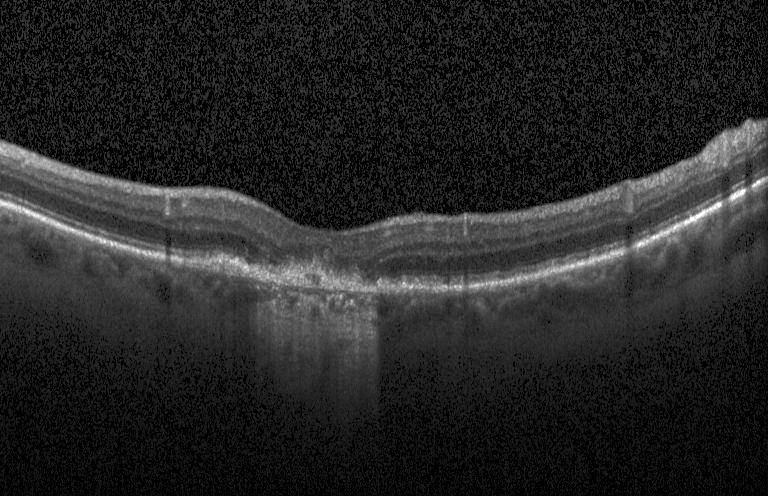
OCT line scan. OCT finding: choroidal neovascularization.